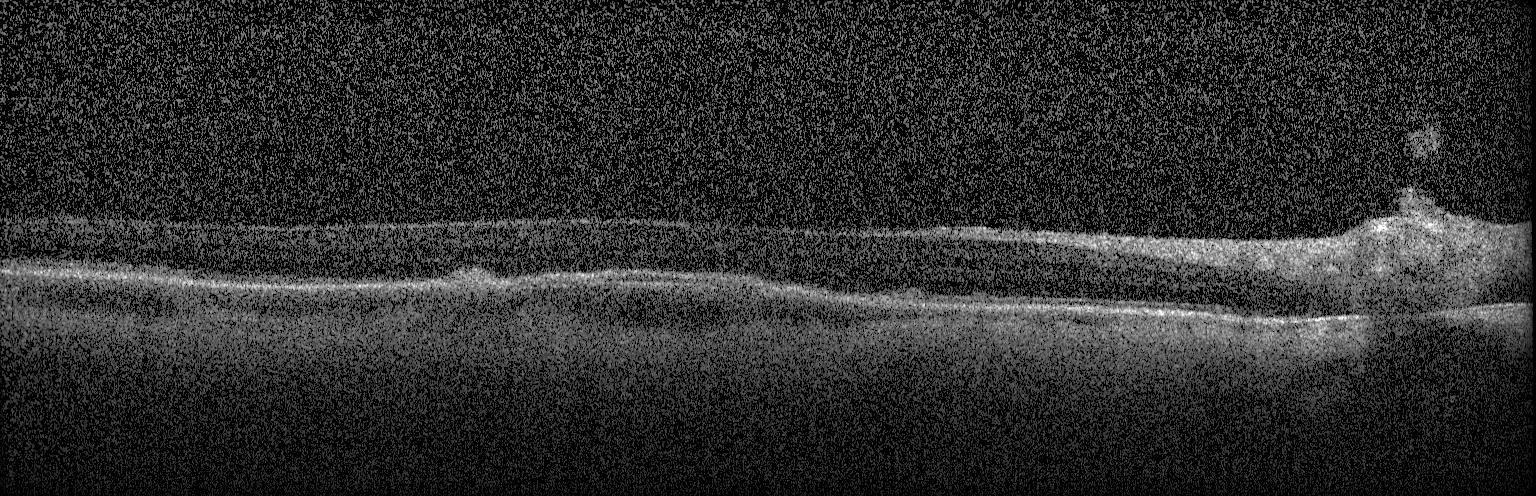
Retinal OCT cross-section; instrument: Heidelberg Spectralis; horizontal scan through the fovea — Dx: a choroidal neovascular membrane.